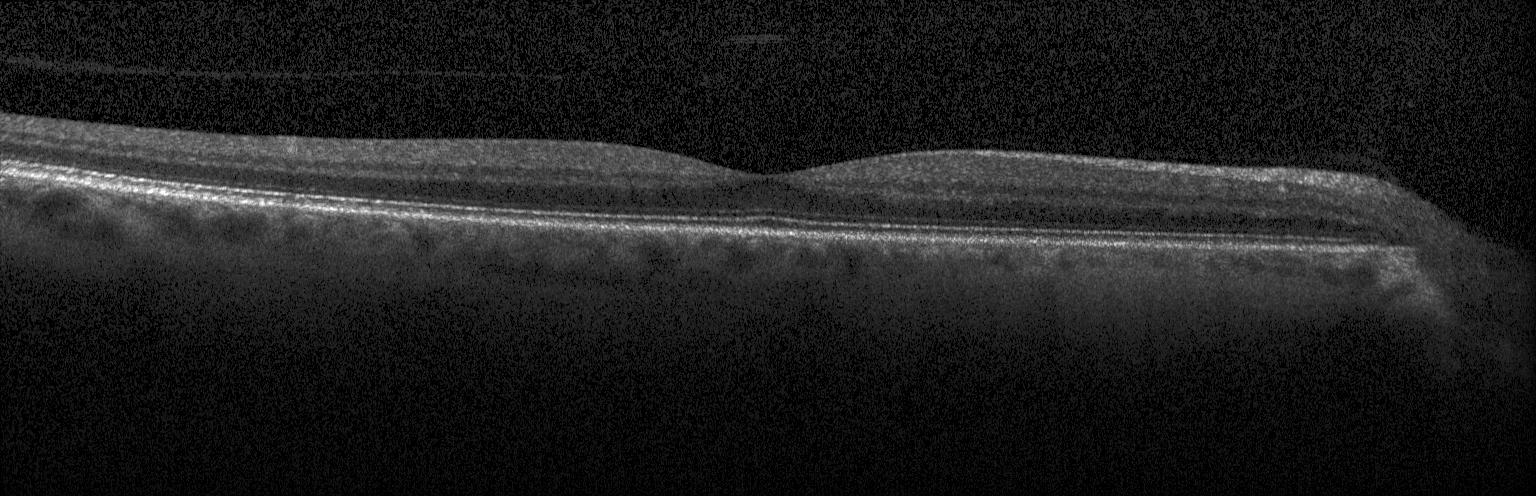 OCT scan showing no CNV, no DME, and no drusen.